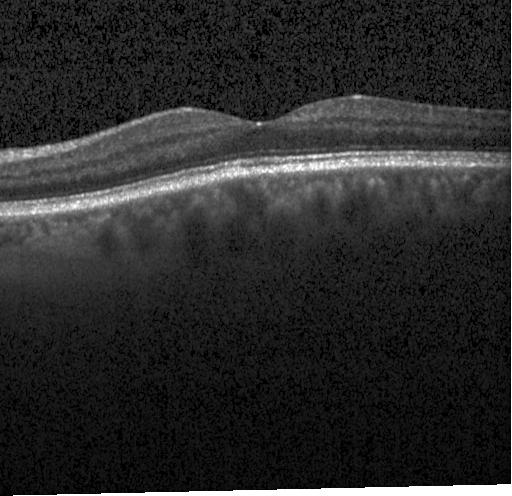 Retinal OCT cross-section. Horizontal scan through the fovea
Dx: neither choroidal neovascularization, diabetic macular edema, nor drusen.